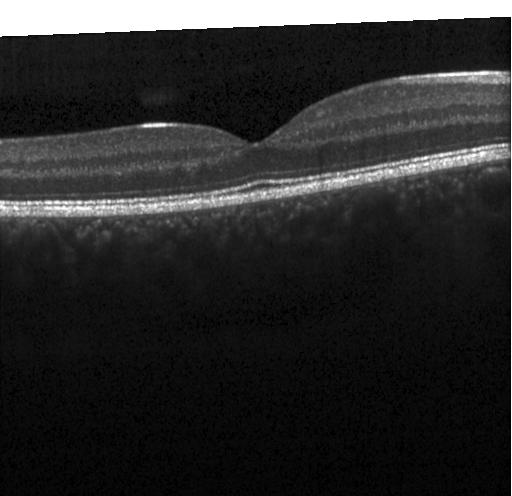

Impression: no evidence of choroidal neovascularization, diabetic macular edema, or drusen.